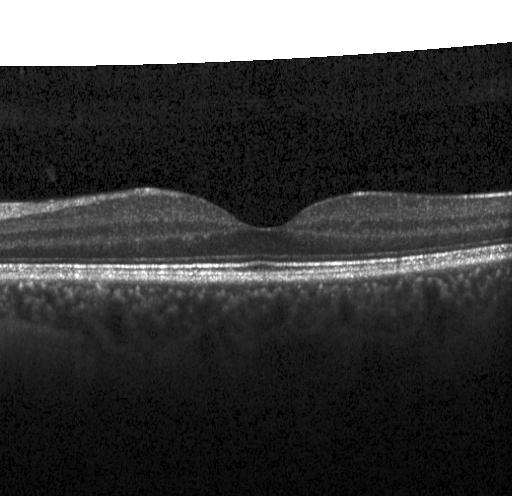 Optical coherence tomography B-scan; spectral-domain OCT; Heidelberg Spectralis OCT system; macular scan — The scan shows no evidence of choroidal neovascularization, diabetic macular edema, or drusen.